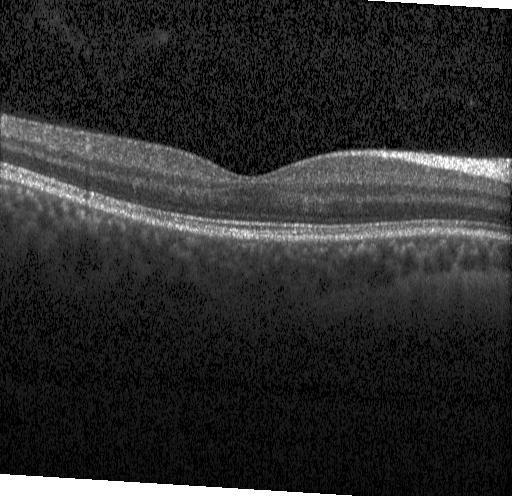

Finding: neither choroidal neovascularization, diabetic macular edema, nor drusen.